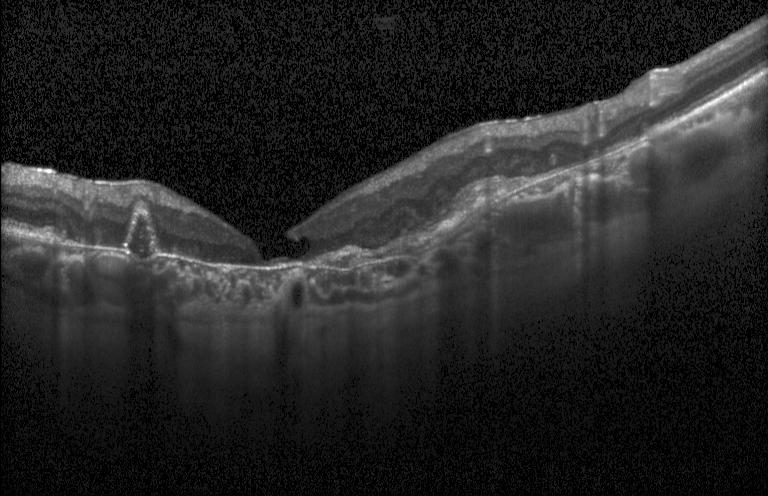

Diagnosis: CNV.